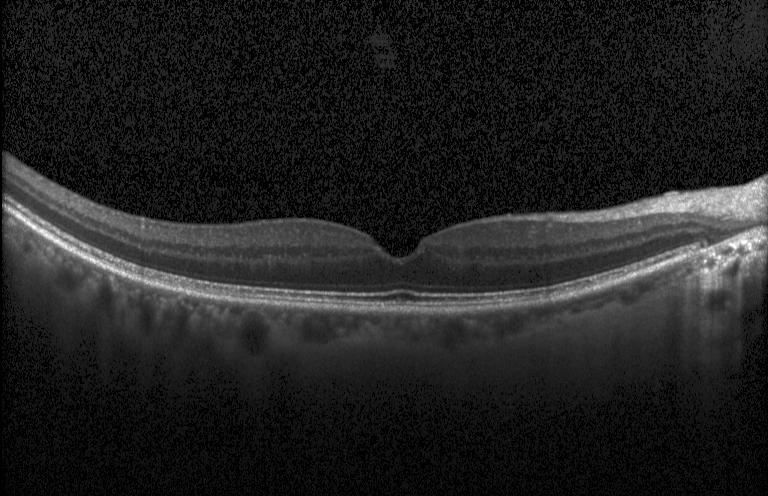

Spectral-domain optical coherence tomography. Macular scan. Optical coherence tomography scan
Diagnosis: no evidence of choroidal neovascularization, diabetic macular edema, or drusen.